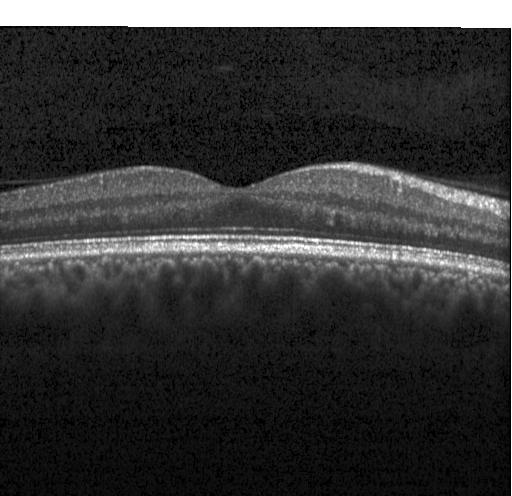 Acquired on a Heidelberg Spectralis; optical coherence tomography B-scan; spectral-domain OCT.
OCT finding: no choroidal neovascularization, diabetic macular edema, or drusen.